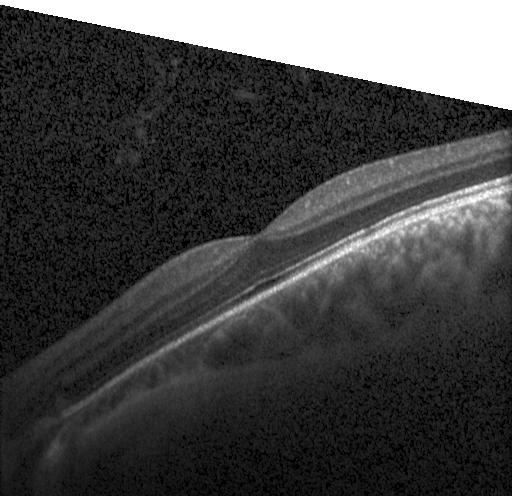
Diagnosis: no evidence of choroidal neovascularization, diabetic macular edema, or drusen.